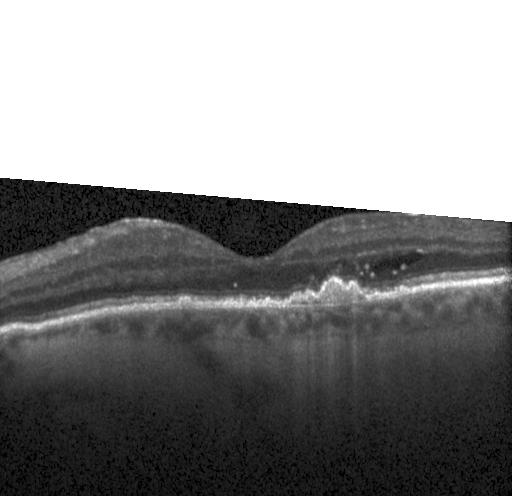
Macular scan, optical coherence tomography scan, spectral-domain OCT, instrument: Heidelberg Spectralis — Drusen.